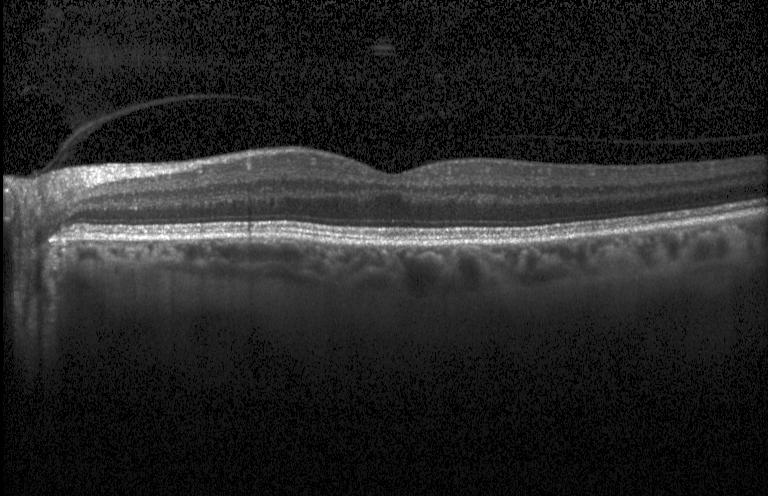
Diagnosis: no choroidal neovascularization, diabetic macular edema, or drusen.